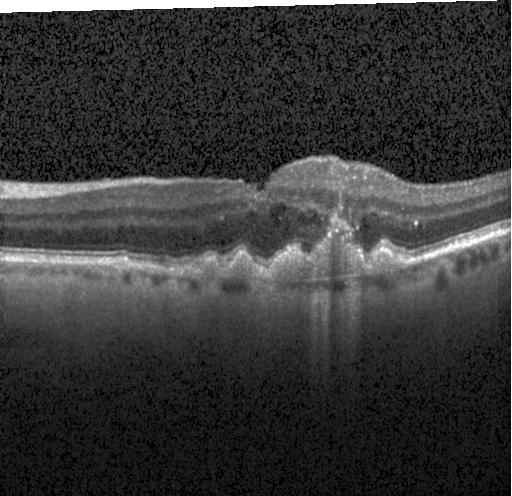 Horizontal scan through the fovea; OCT line scan
Impression: CNV.